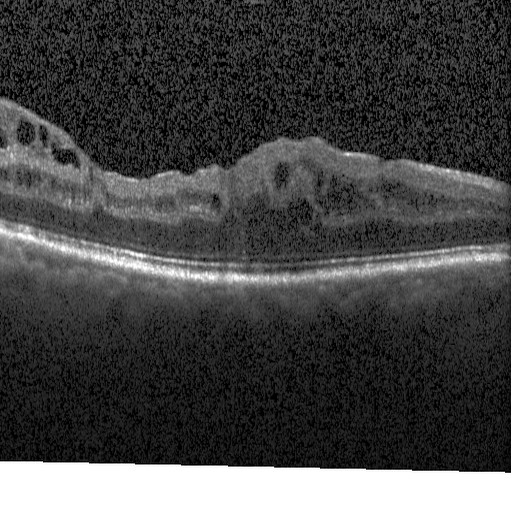
This B-scan demonstrates diabetic macular edema.